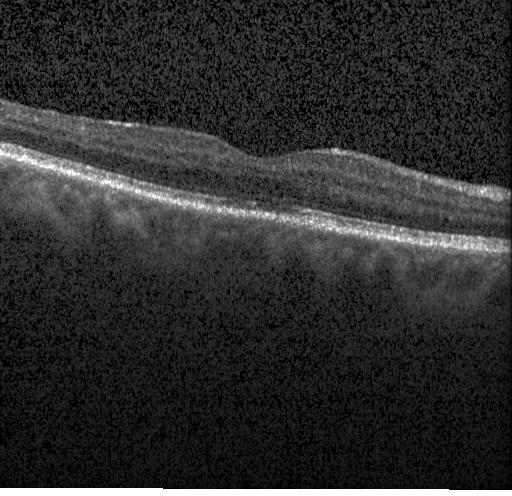

Spectral-domain optical coherence tomography · optical coherence tomography scan — Diagnosis: no CNV, no DME, and no drusen.